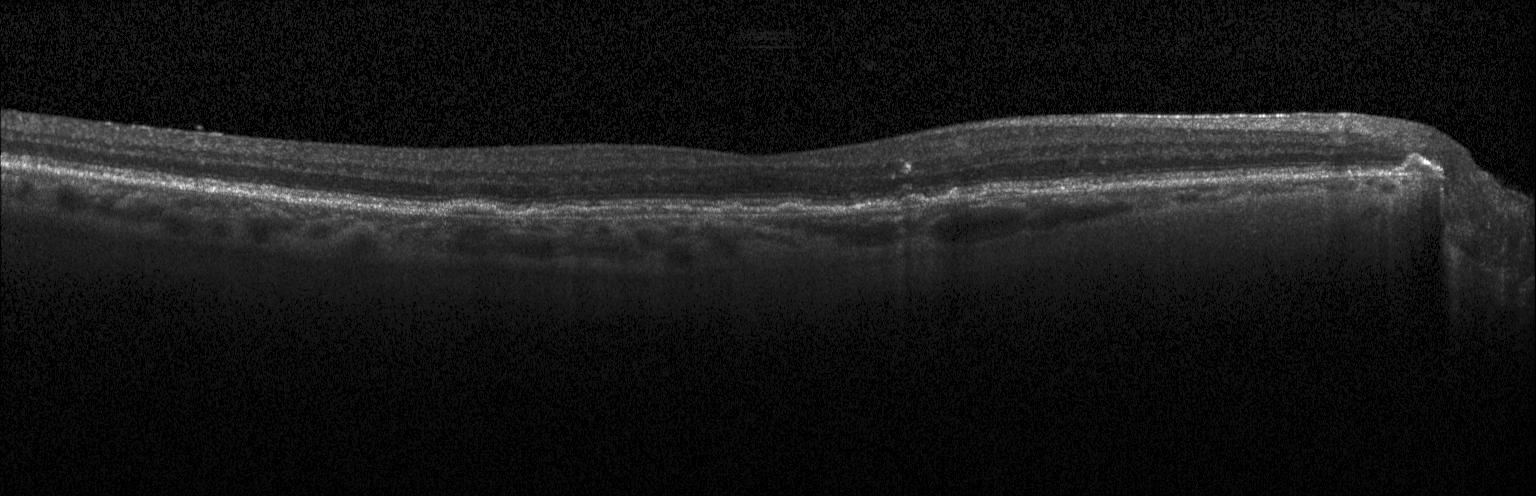

Finding: a choroidal neovascular membrane.